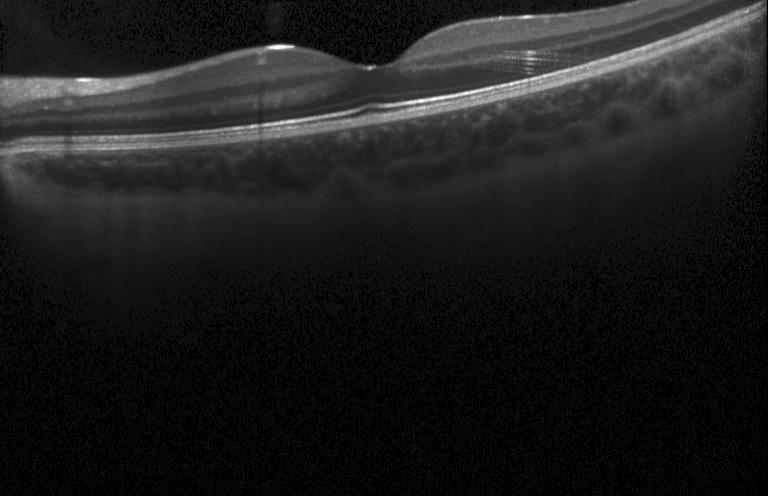 Spectral-domain optical coherence tomography, OCT B-scan, fovea-centered
OCT finding: no choroidal neovascularization, diabetic macular edema, or drusen.